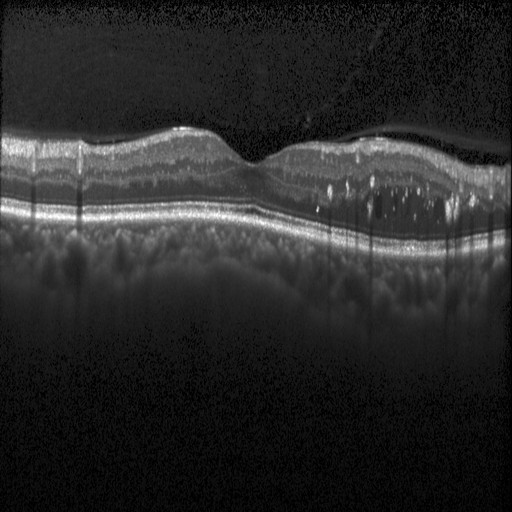

The scan shows diabetic macular edema (DME).